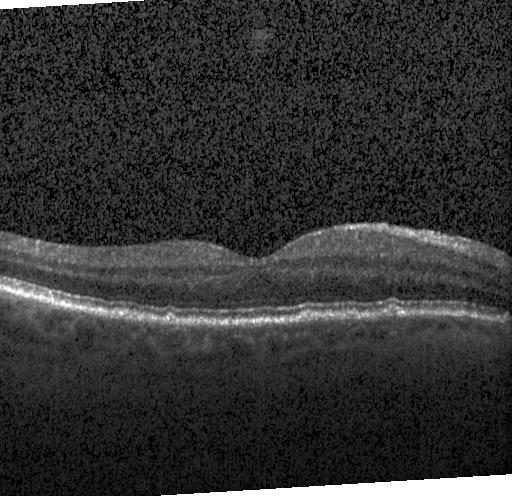 Instrument: Heidelberg Spectralis; optical coherence tomography B-scan
Impression: multiple drusen.